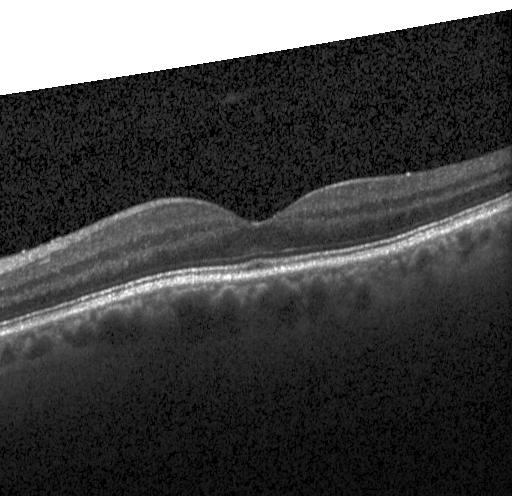

Macular OCT: no choroidal neovascularization, no diabetic macular edema, and no drusen.